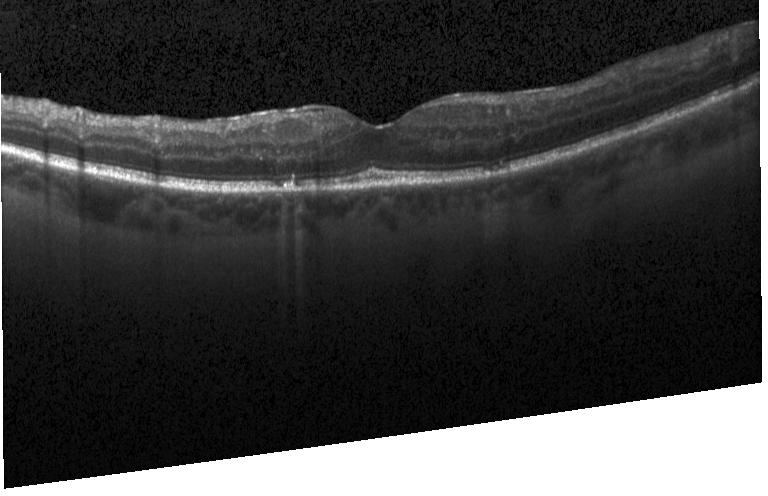 Dx: diabetic macular edema (DME).